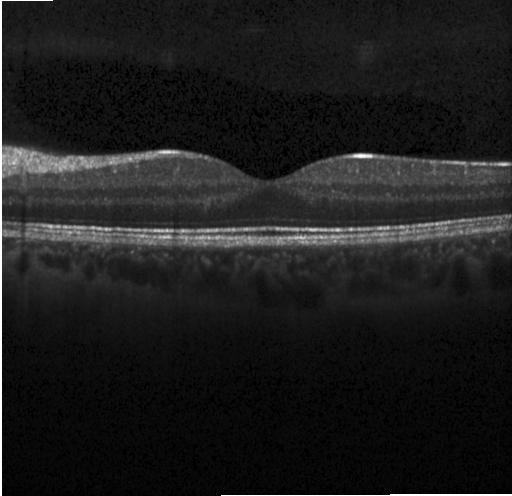
Diagnosis: neither choroidal neovascularization, diabetic macular edema, nor drusen.